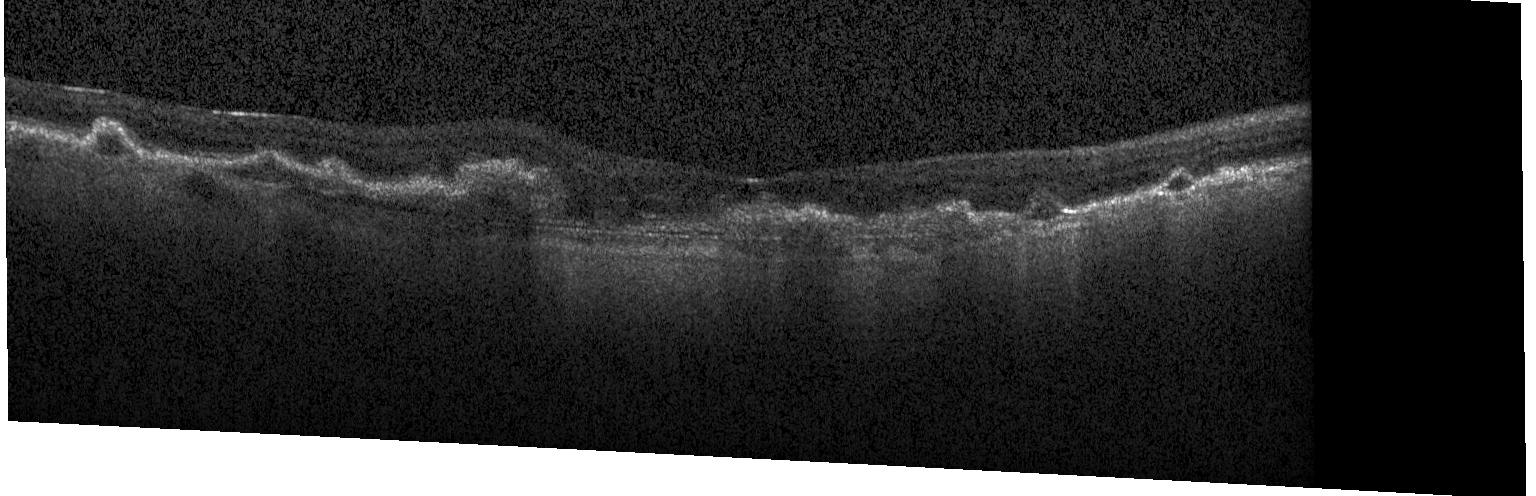 Optical coherence tomography scan · SD-OCT · instrument: Heidelberg Spectralis — OCT finding: CNV.